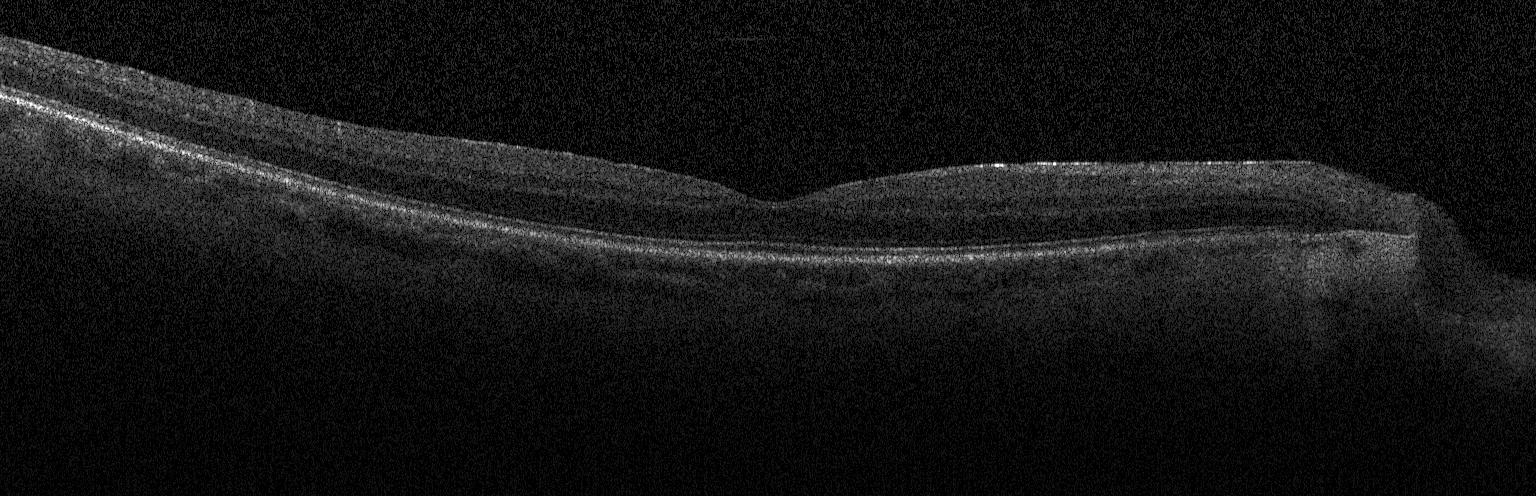 Macular scan, retinal OCT cross-section.
This B-scan demonstrates neither CNV, DME, nor drusen.